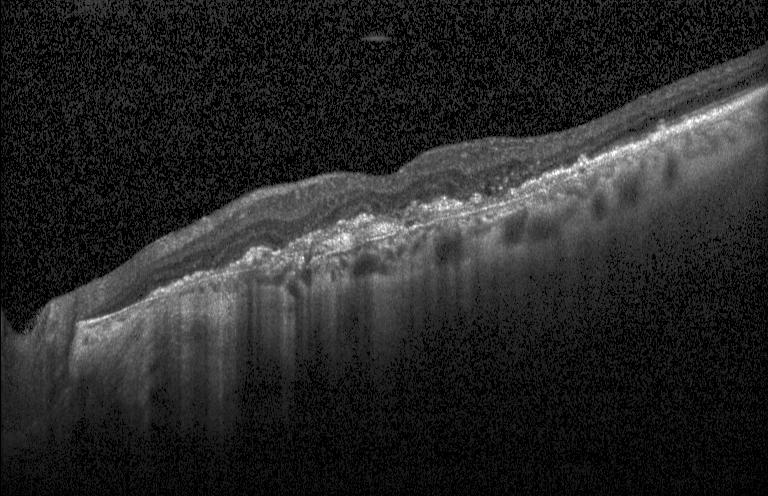
Dx: a choroidal neovascular membrane.